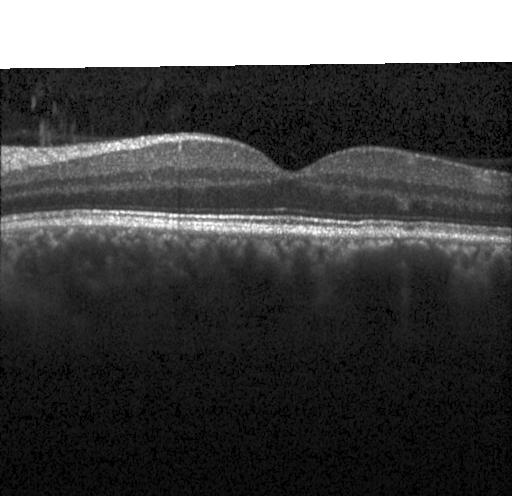

Macular OCT demonstrating no choroidal neovascularization, no diabetic macular edema, and no drusen.